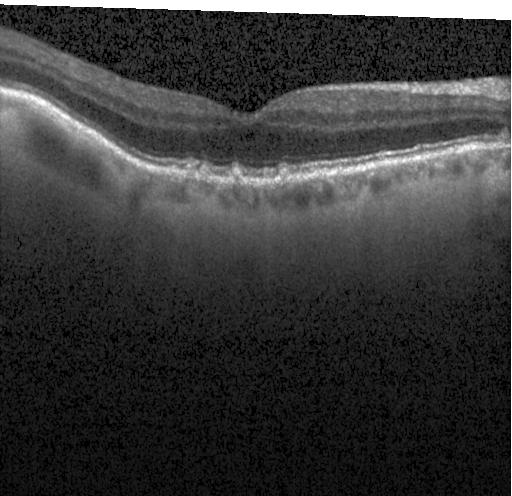

Heidelberg Spectralis OCT system; retinal OCT cross-section; macular scan; spectral-domain optical coherence tomography.
Macular OCT: drusen.